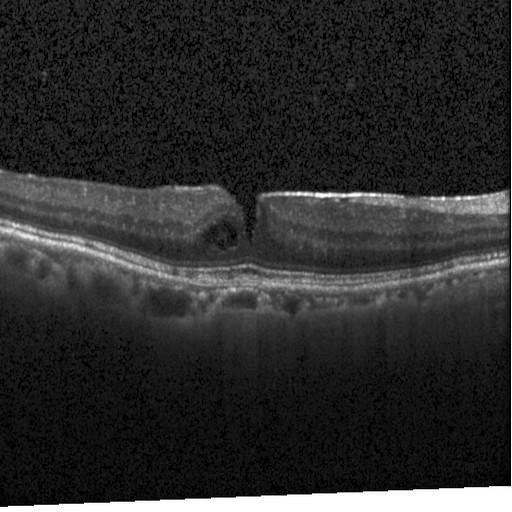 Assessment: diabetic macular edema.